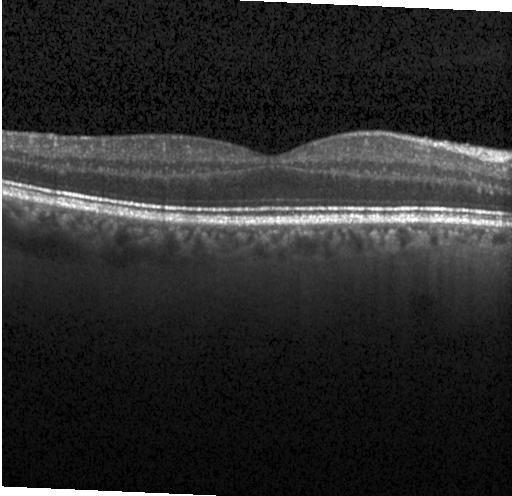 Diagnosis: no evidence of CNV, DME, or drusen.